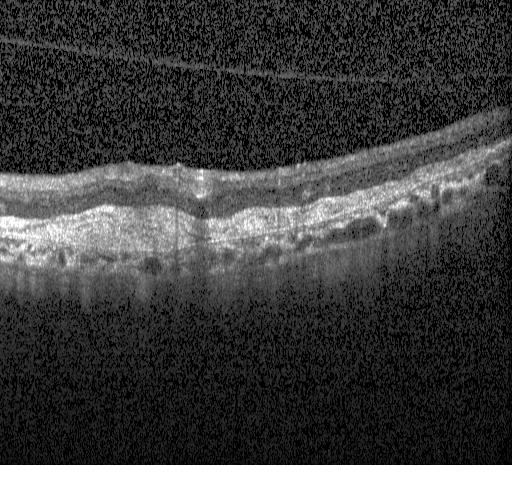 The scan shows choroidal neovascularization (CNV).